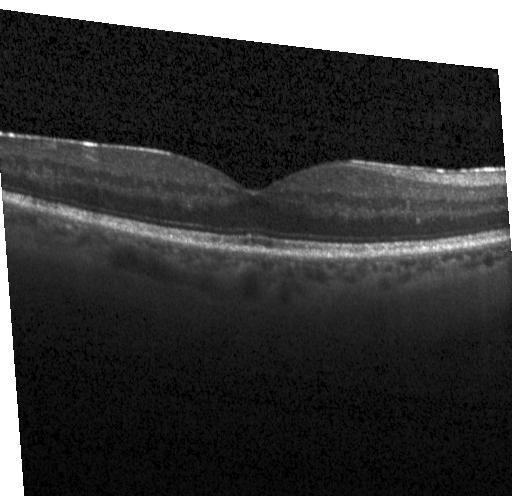

Optical coherence tomography B-scan · macular scan. Assessment: neither CNV, DME, nor drusen.